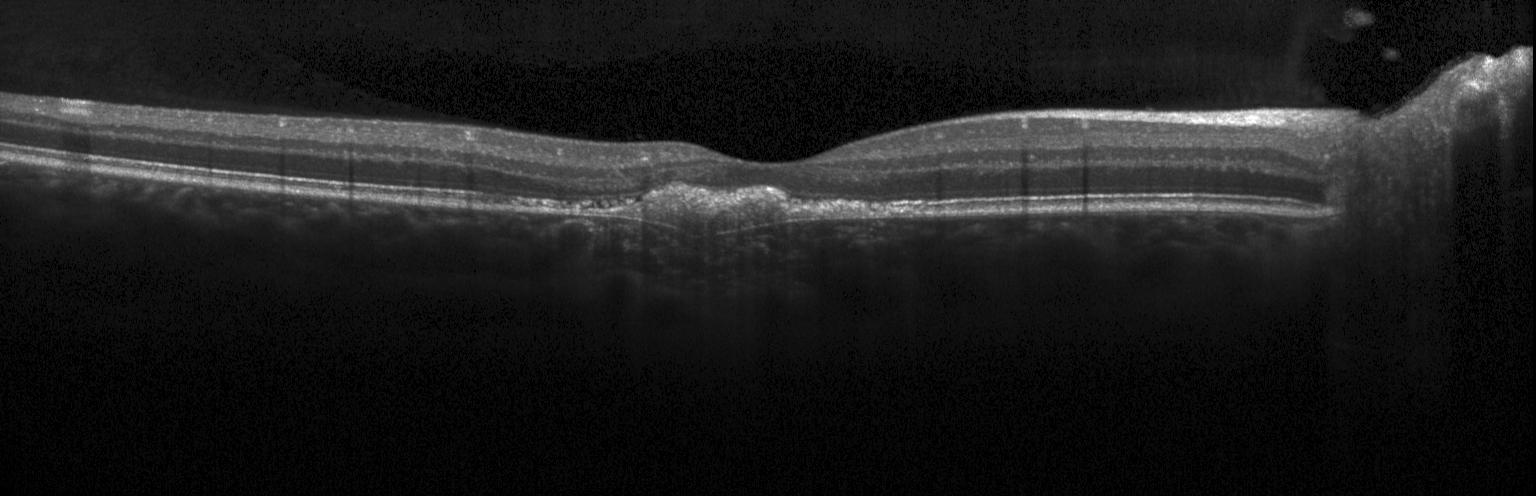 Diagnosis: a choroidal neovascular membrane.